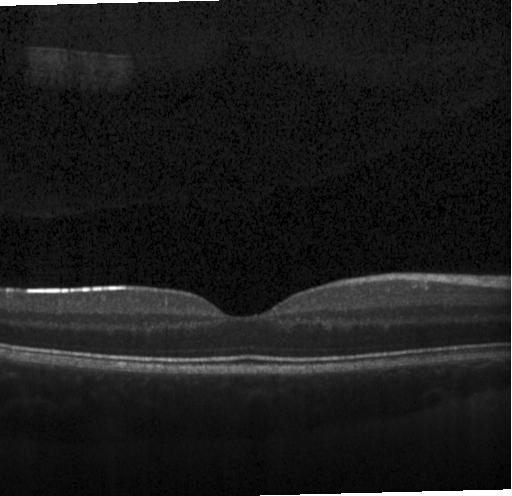 OCT B-scan, through the macula, instrument: Heidelberg Spectralis, spectral-domain optical coherence tomography
Finding: no choroidal neovascularization, diabetic macular edema, or drusen.